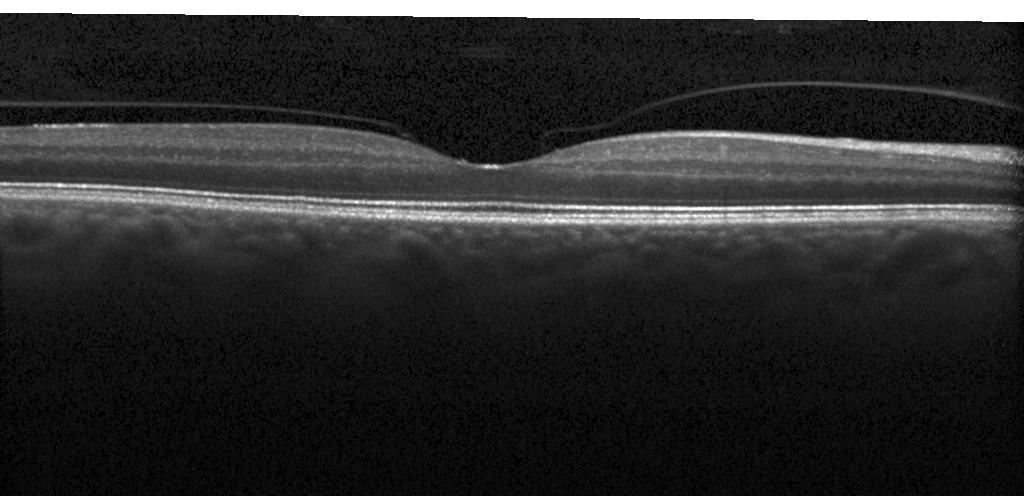

Through the macula. Optical coherence tomography B-scan. Heidelberg Spectralis OCT system. Spectral-domain optical coherence tomography. Diagnosis: no CNV, no DME, and no drusen.